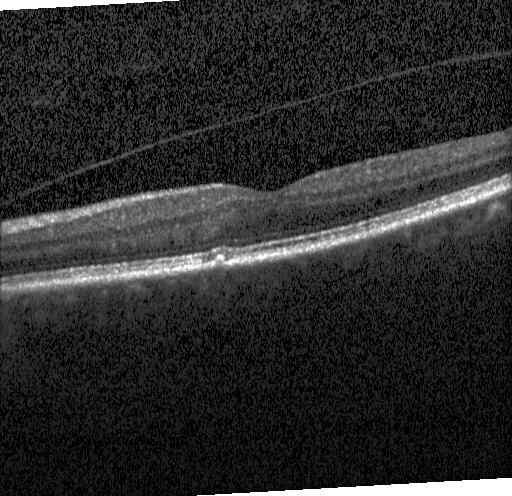
Macular OCT: sub-RPE drusenoid deposits.